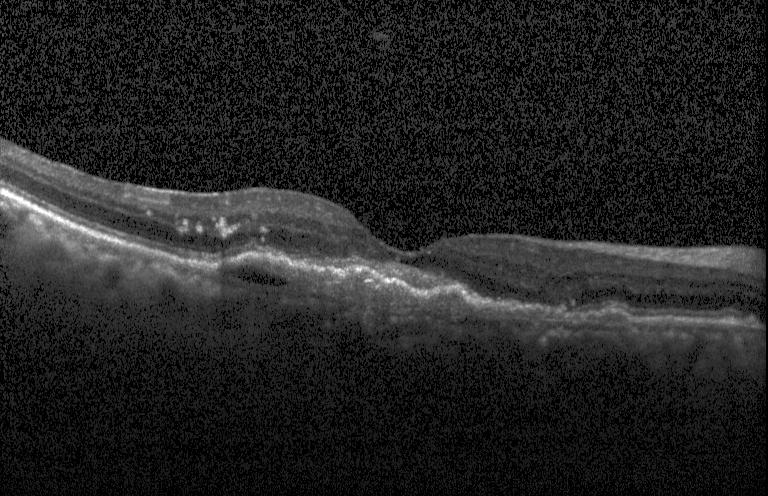 Assessment: a choroidal neovascular membrane.